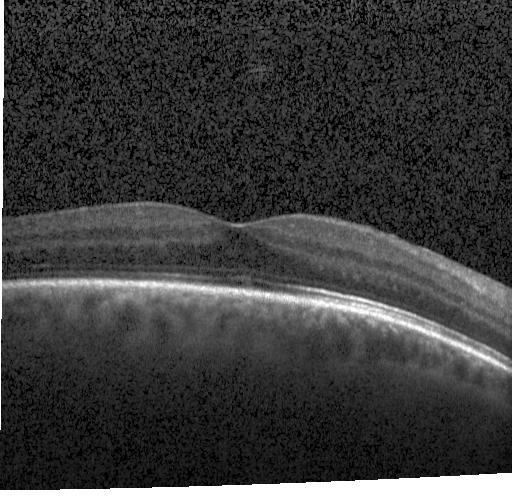

OCT finding: no choroidal neovascularization, no diabetic macular edema, and no drusen.